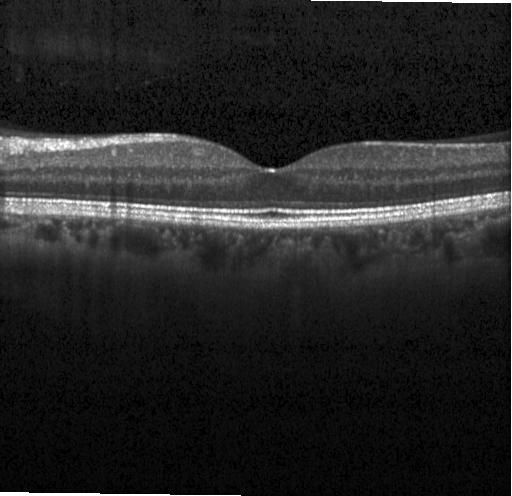 OCT line scan. Fovea-centered. Heidelberg Spectralis OCT system
No evidence of CNV, DME, or drusen.